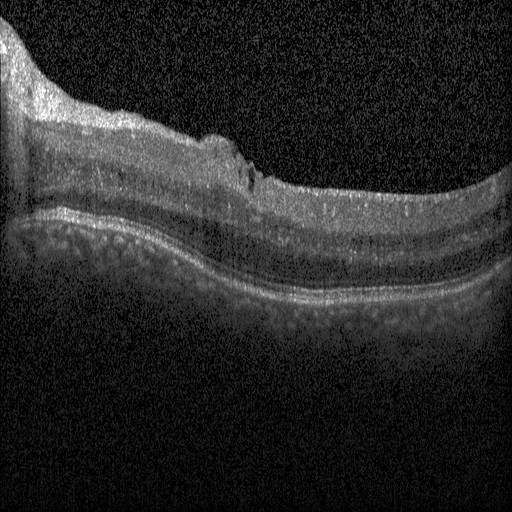 Retinal OCT cross-section, spectral-domain optical coherence tomography, instrument: Heidelberg Spectralis — Assessment: DME.